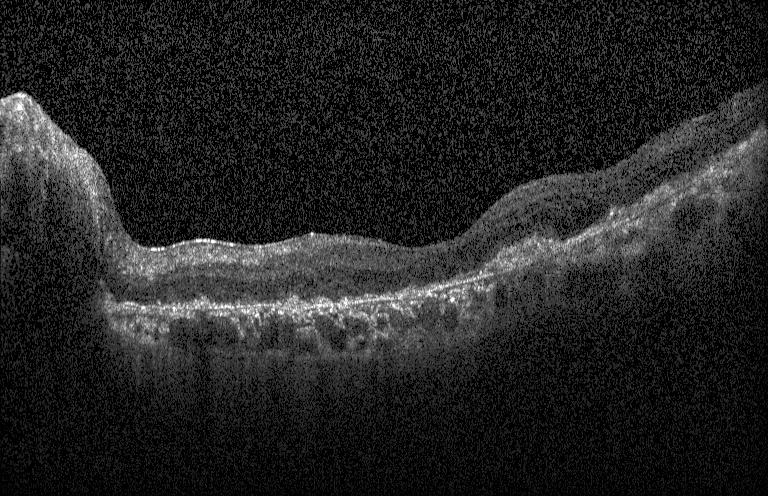
Finding: choroidal neovascularization.